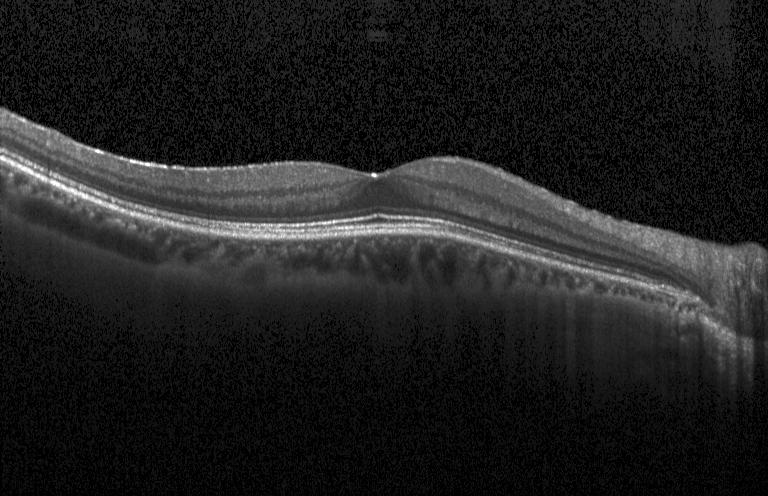

Optical coherence tomography B-scan — Finding: no CNV, DME, or drusen.